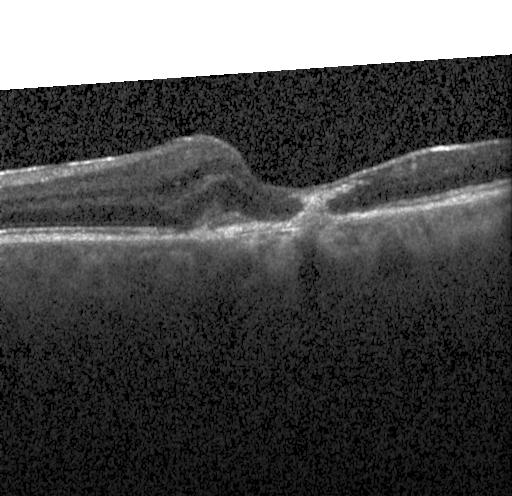

Diagnosis: CNV.